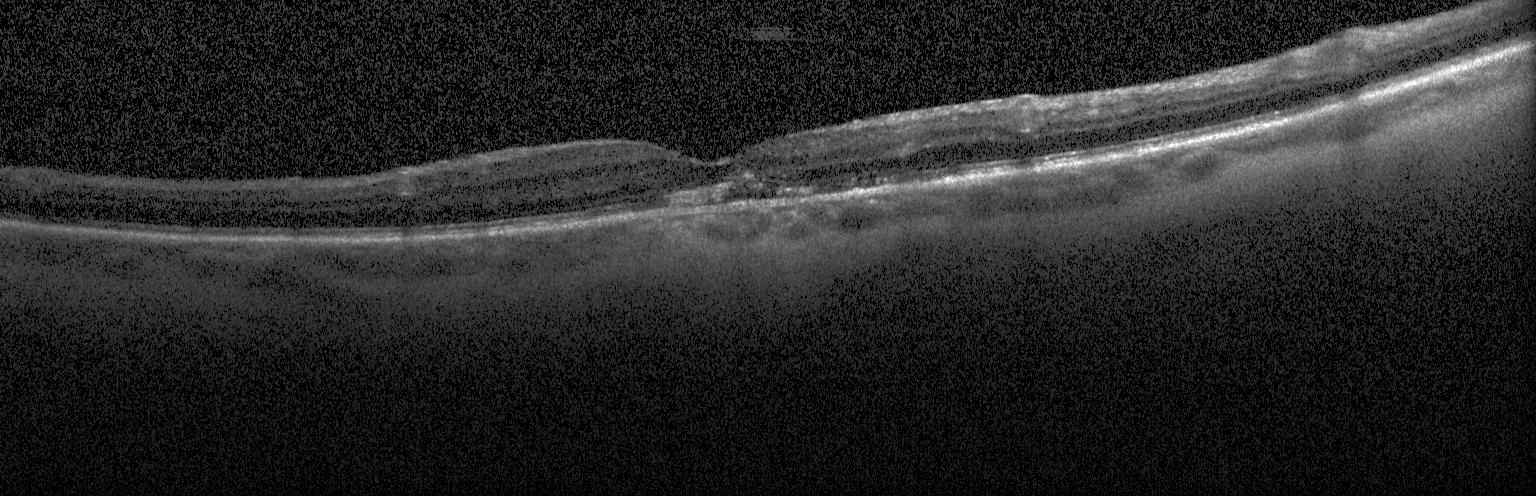

Retinal OCT cross-section.
The scan shows a choroidal neovascular membrane.